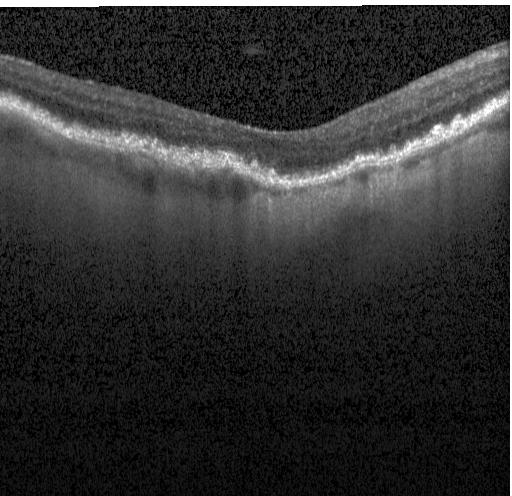

Centered on the fovea. Optical coherence tomography scan
Macular OCT: a choroidal neovascular membrane.